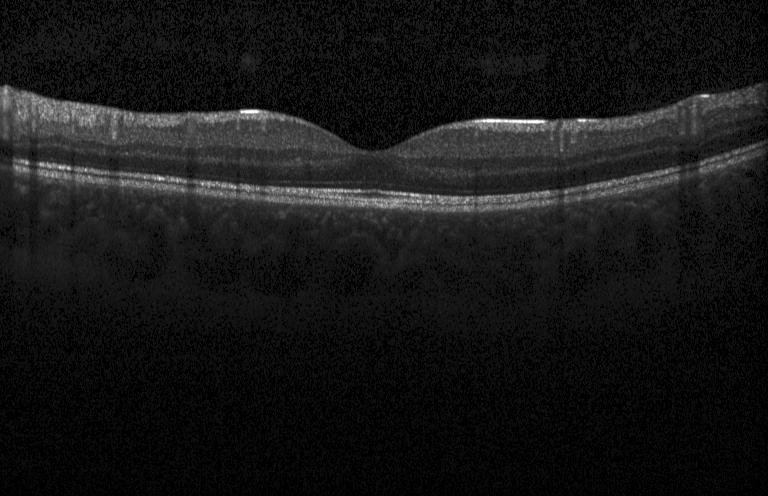

Spectral-domain optical coherence tomography · macular scan · acquired on a Heidelberg Spectralis · OCT line scan — Dx: no choroidal neovascularization, diabetic macular edema, or drusen.